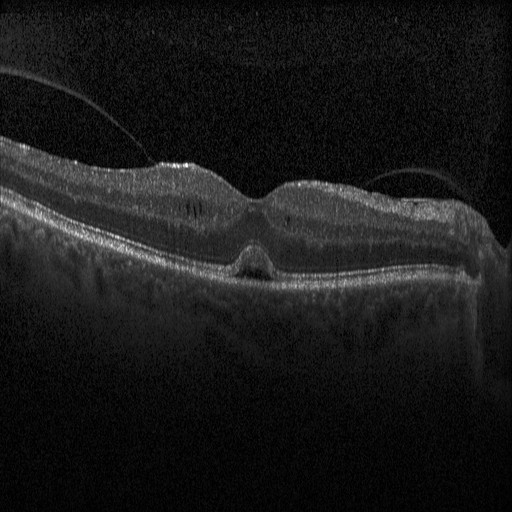

Retinal OCT cross-section; fovea-centered; SD-OCT; Heidelberg Spectralis. DME.